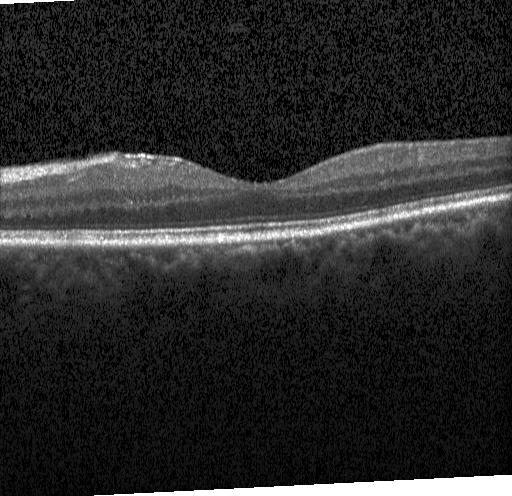 OCT B-scan showing no evidence of choroidal neovascularization, diabetic macular edema, or drusen.